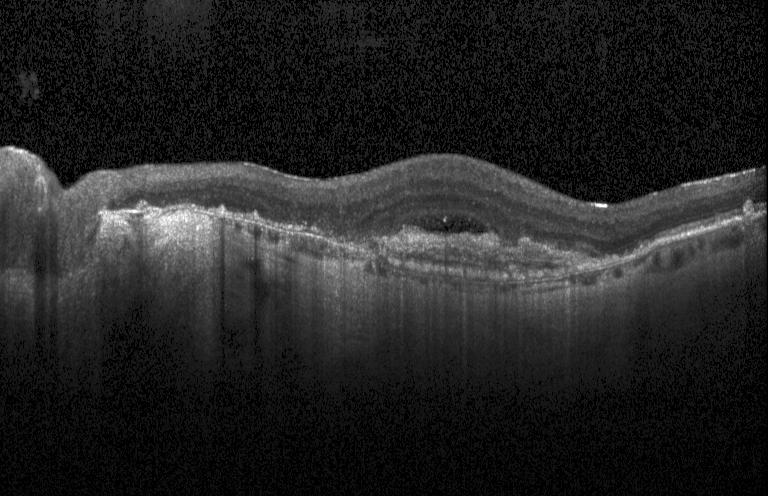 SD-OCT, retinal OCT B-scan, Heidelberg Spectralis OCT system — This B-scan demonstrates a choroidal neovascular membrane.